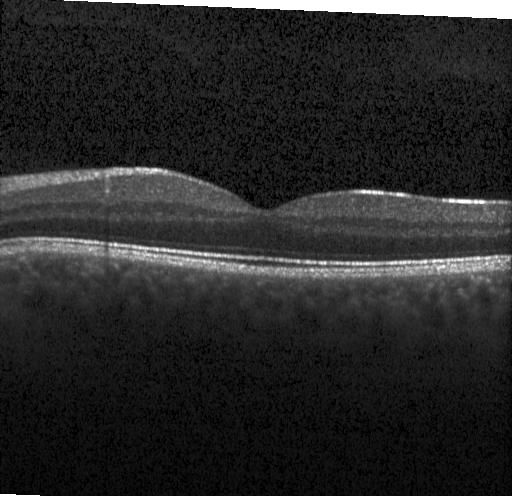 Dx: no choroidal neovascularization, diabetic macular edema, or drusen.